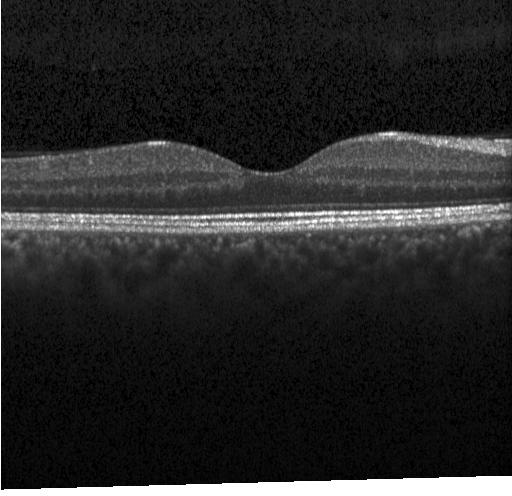 The scan shows no choroidal neovascularization, no diabetic macular edema, and no drusen.